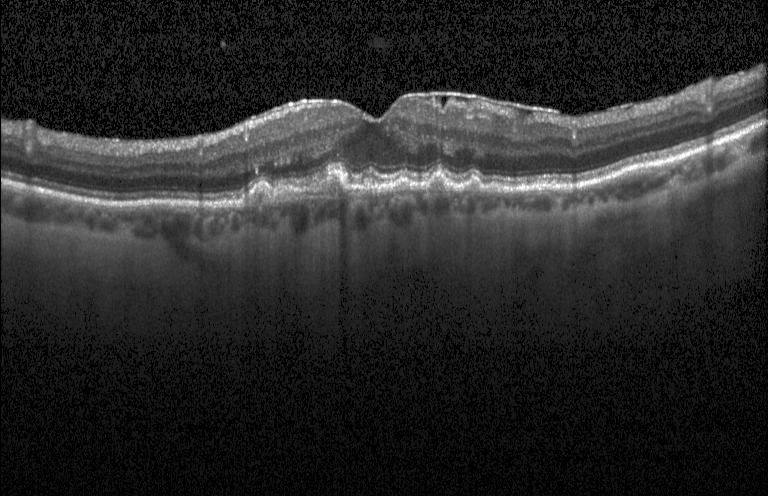

Optical coherence tomography scan; instrument: Heidelberg Spectralis.
OCT finding: multiple drusen.